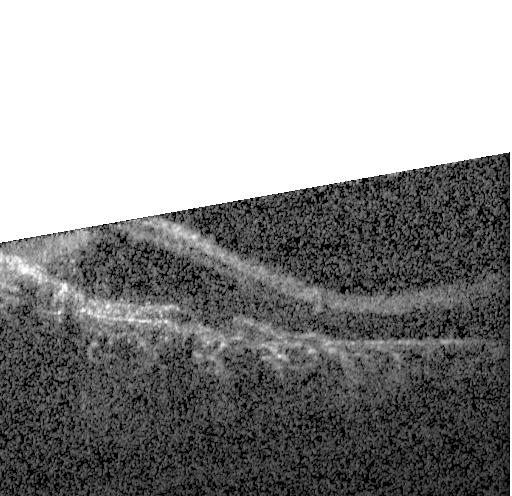

OCT B-scan.
Finding: a choroidal neovascular membrane.